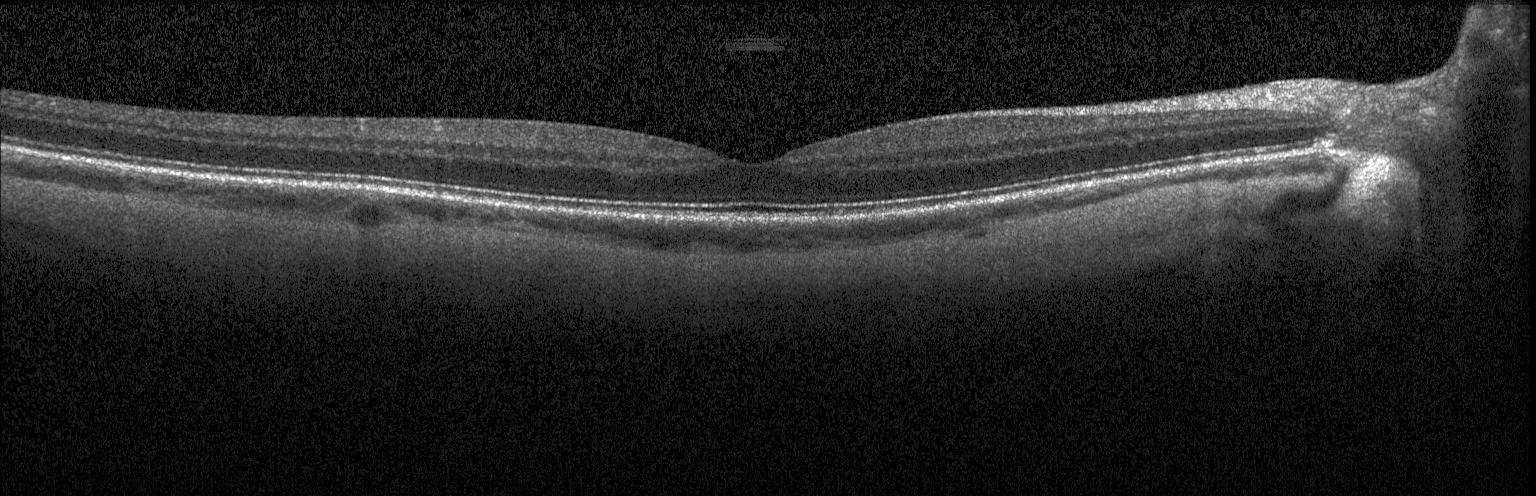

SD-OCT, horizontal scan through the fovea, optical coherence tomography B-scan.
The scan shows no evidence of choroidal neovascularization, diabetic macular edema, or drusen.